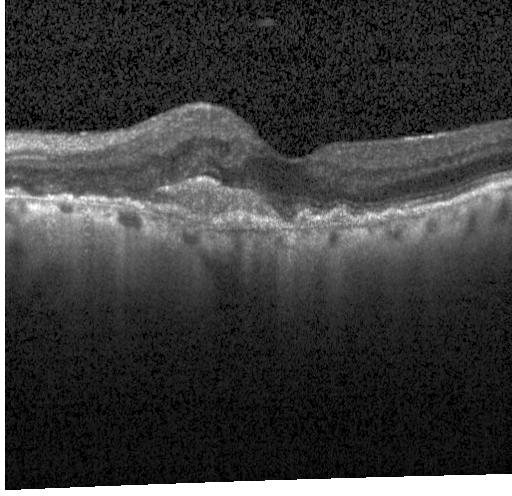 OCT line scan — Finding: choroidal neovascularization (CNV).